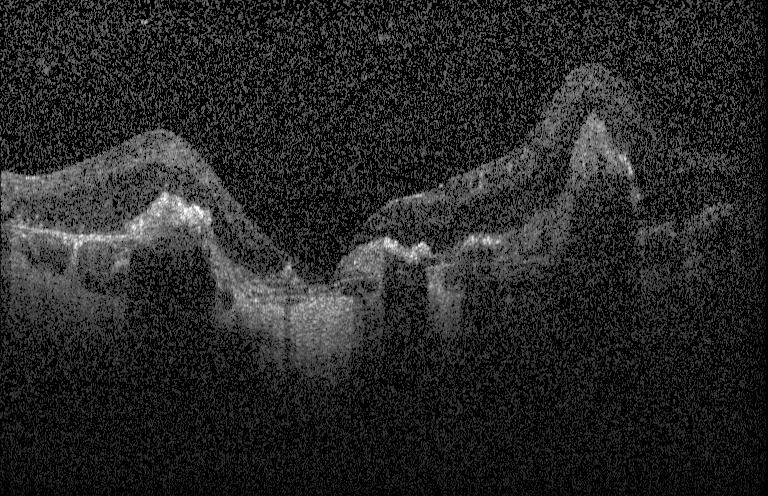

OCT line scan. Spectral-domain optical coherence tomography — This B-scan demonstrates a choroidal neovascular membrane.